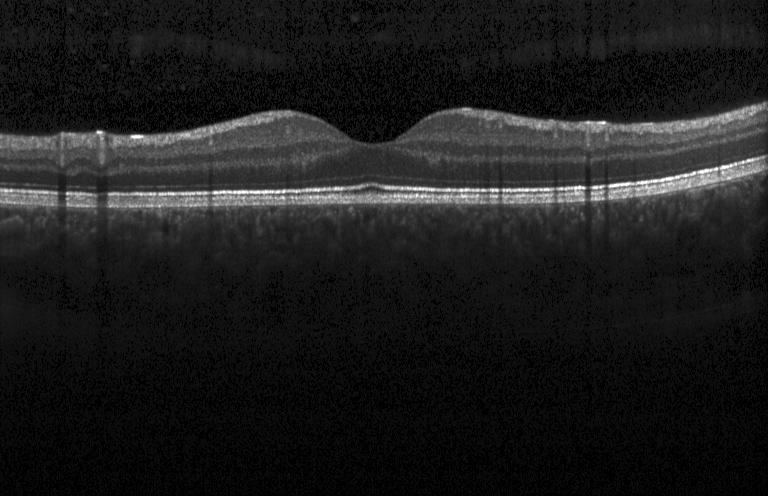
Macular OCT demonstrating no evidence of choroidal neovascularization, diabetic macular edema, or drusen.